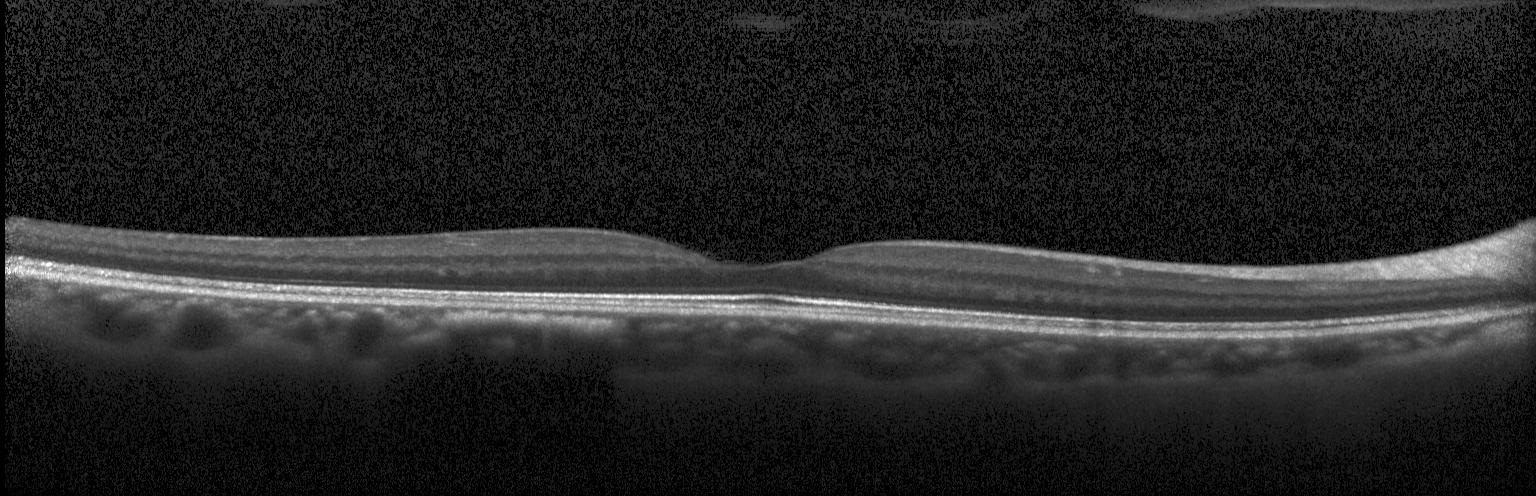

OCT finding: no CNV, DME, or drusen.